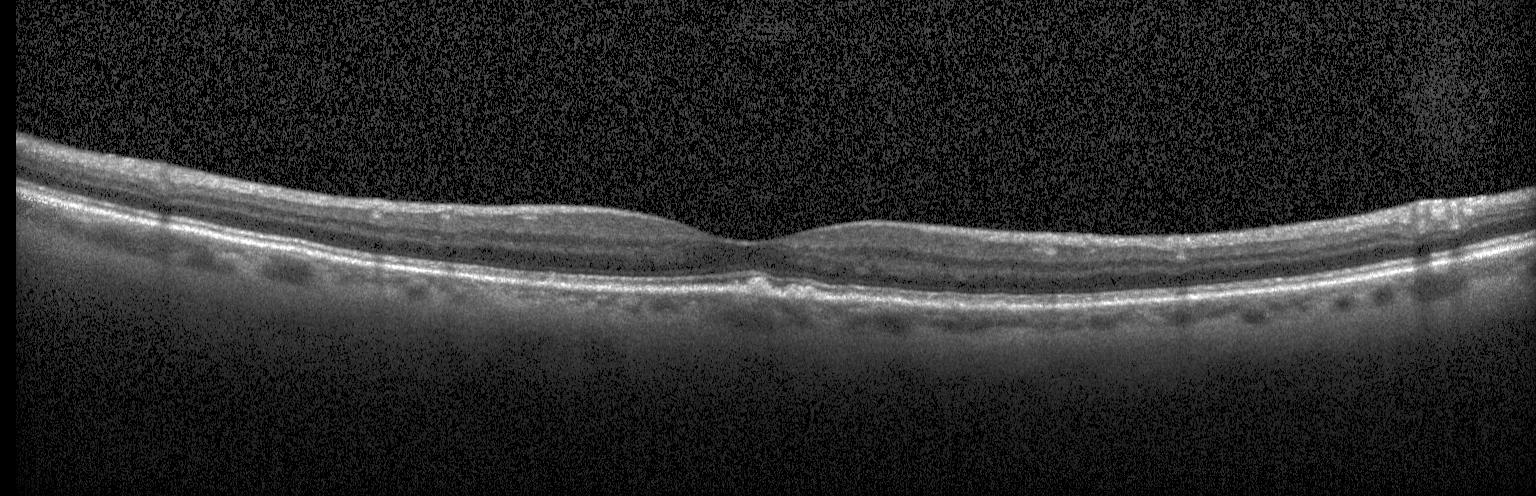
Horizontal scan through the fovea. Optical coherence tomography scan.
Macular OCT: sub-RPE drusenoid deposits.